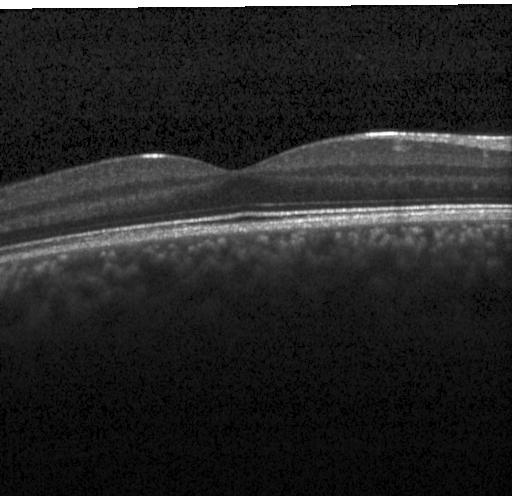 Retinal OCT cross-section.
Finding: neither choroidal neovascularization, diabetic macular edema, nor drusen.